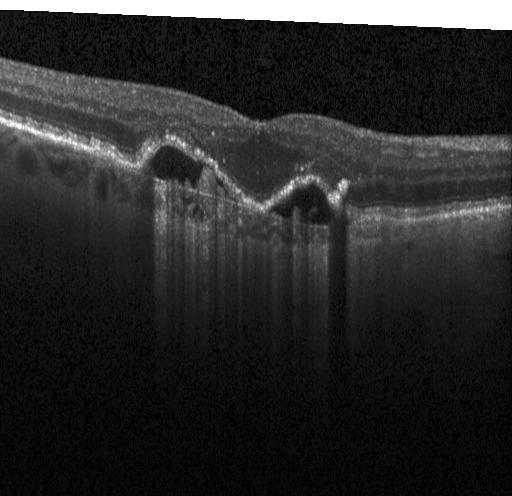

Optical coherence tomography scan, instrument: Heidelberg Spectralis, SD-OCT, through the macula — Diagnosis: a choroidal neovascular membrane.